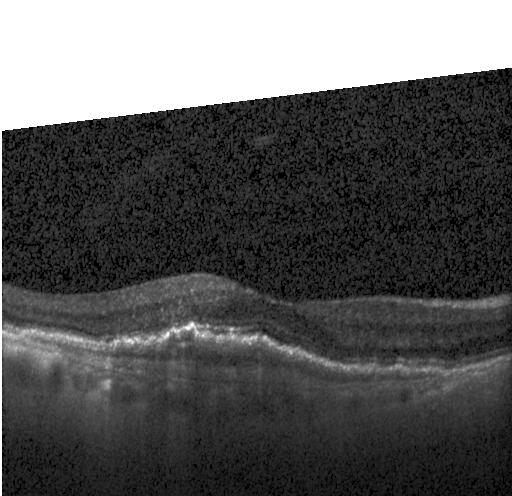 OCT B-scan.
OCT finding: a choroidal neovascular membrane.